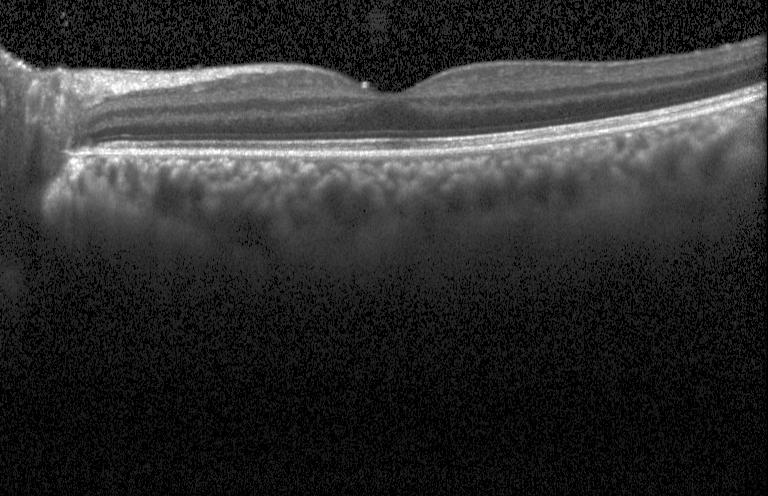

Horizontal scan through the fovea; acquired on a Heidelberg Spectralis; OCT B-scan; spectral-domain optical coherence tomography. Macular OCT: no evidence of choroidal neovascularization, diabetic macular edema, or drusen.